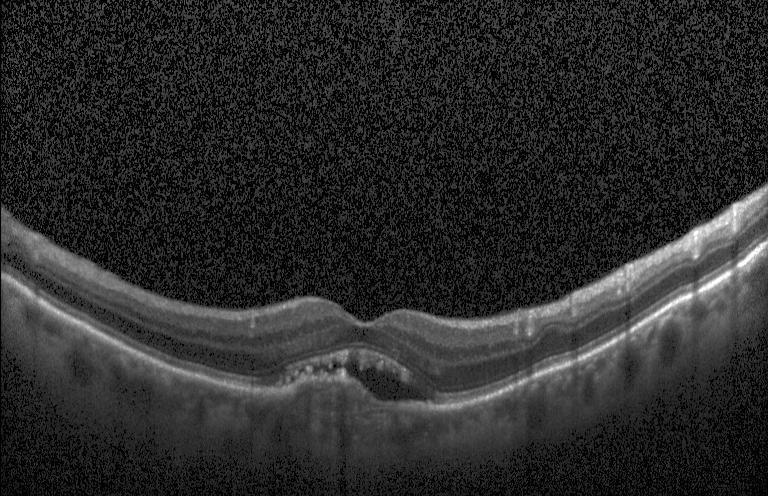

Centered on the fovea. Heidelberg Spectralis. OCT line scan. Spectral-domain OCT — This B-scan demonstrates choroidal neovascularization (CNV).